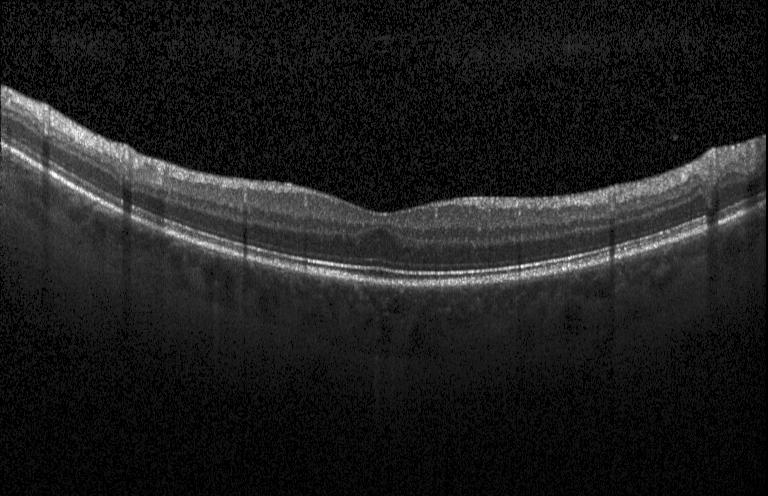

Retinal OCT cross-section. Spectral-domain optical coherence tomography. Assessment: neither CNV, DME, nor drusen.